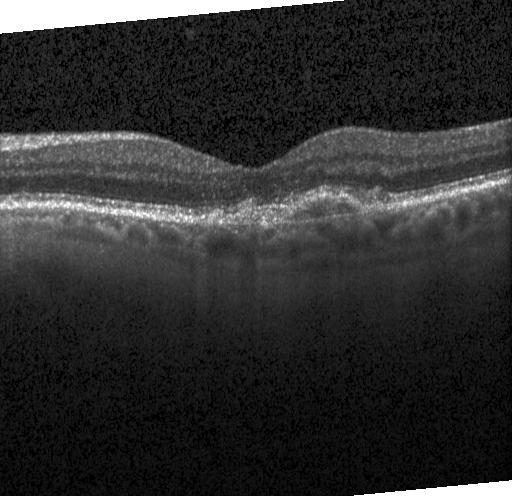
Retinal OCT cross-section, horizontal scan through the fovea.
A choroidal neovascular membrane.